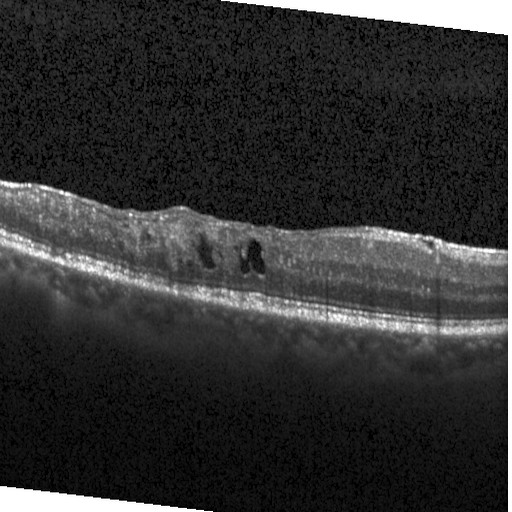 Optical coherence tomography scan — OCT finding: DME.